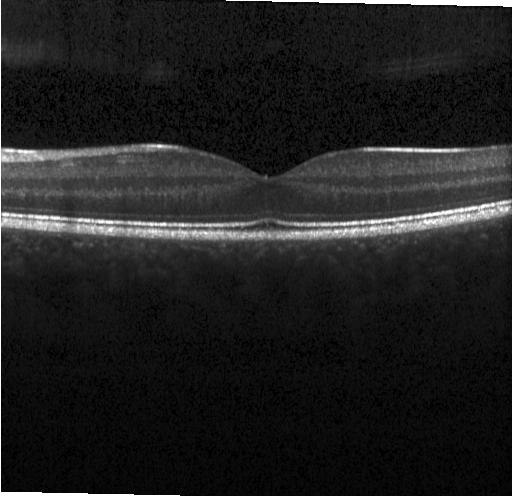

Heidelberg Spectralis OCT system · retinal OCT B-scan · spectral-domain OCT
This B-scan demonstrates no choroidal neovascularization, diabetic macular edema, or drusen.